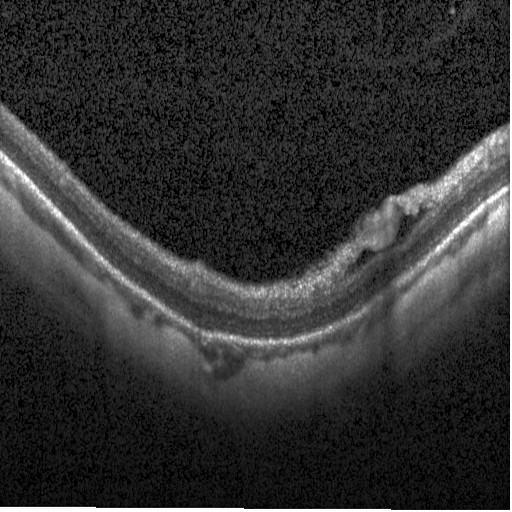
Spectral-domain OCT, fovea-centered, OCT B-scan, acquired on a Heidelberg Spectralis. Macular OCT: diabetic macular edema.